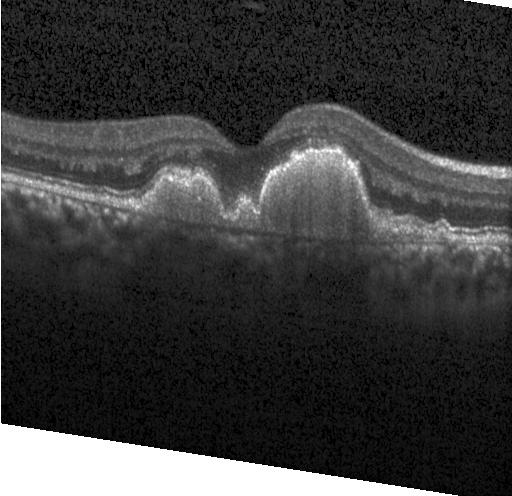 OCT B-scan showing drusen.